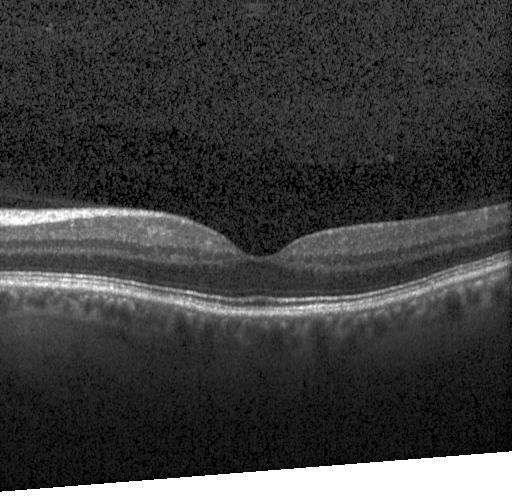

Optical coherence tomography B-scan. Heidelberg Spectralis.
Dx: no evidence of choroidal neovascularization, diabetic macular edema, or drusen.